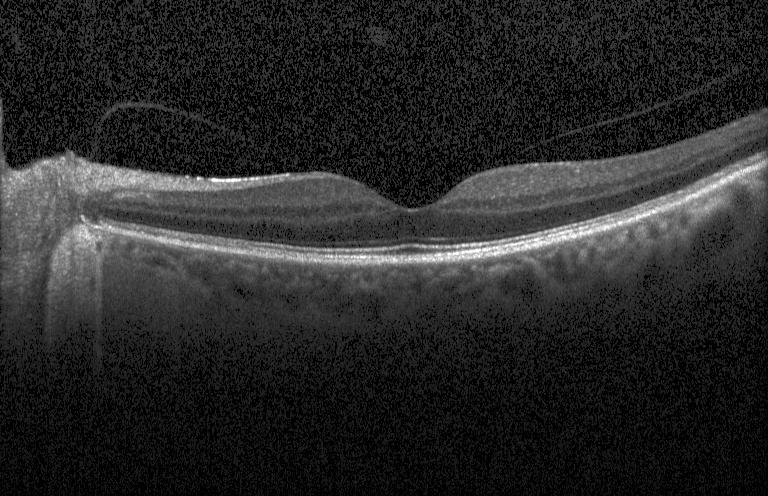
Impression: no choroidal neovascularization, diabetic macular edema, or drusen.